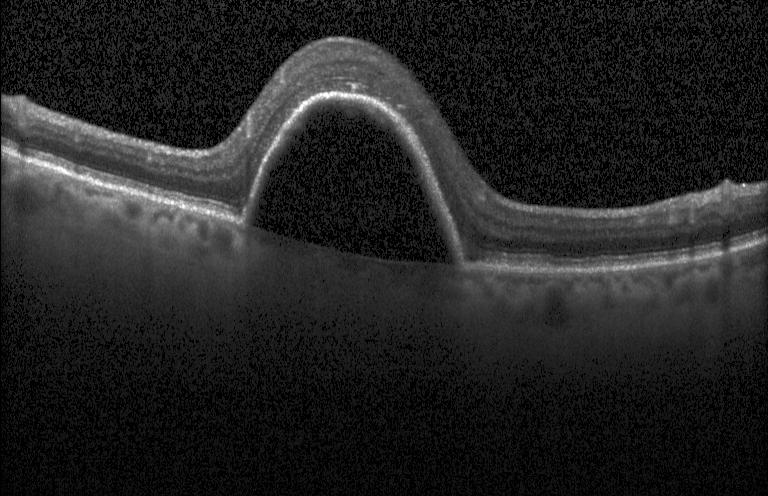 Finding: a choroidal neovascular membrane.